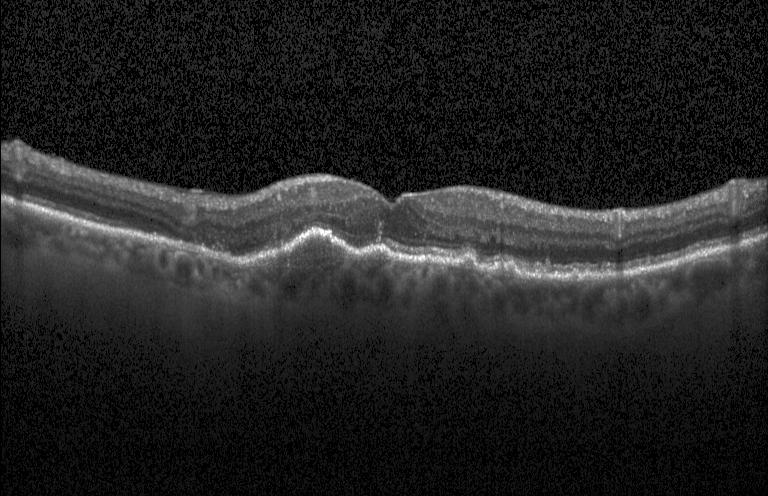 Retinal OCT B-scan
Diagnosis: a choroidal neovascular membrane.